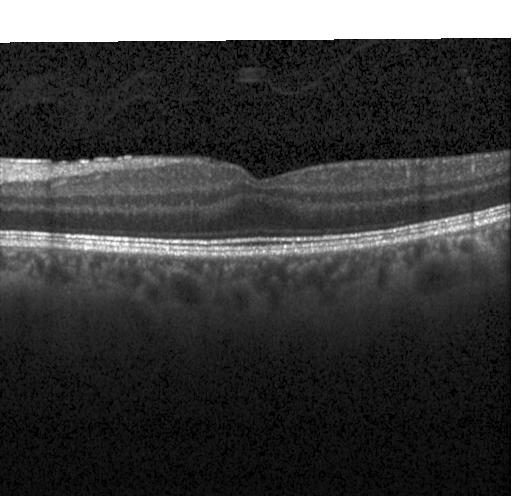 Retinal OCT cross-section — Macular OCT: neither choroidal neovascularization, diabetic macular edema, nor drusen.